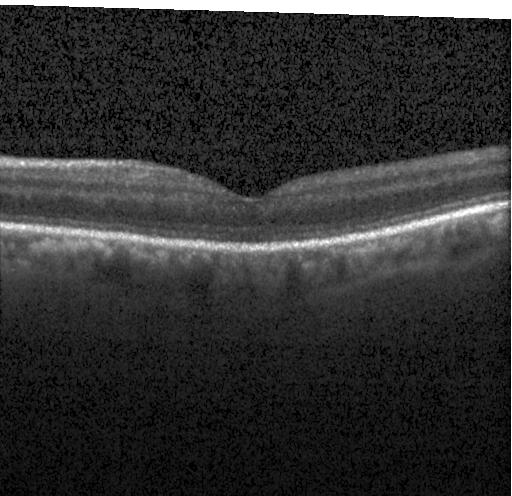
Heidelberg Spectralis. Centered on the fovea. Optical coherence tomography scan. Macular OCT: no choroidal neovascularization, no diabetic macular edema, and no drusen.